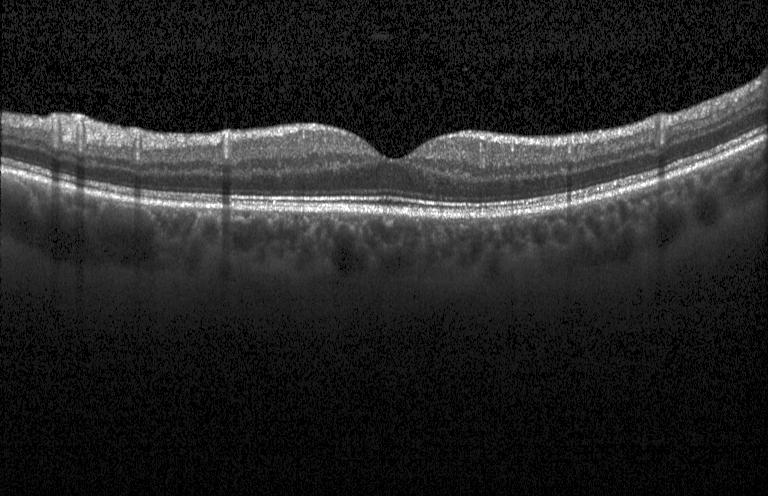

Retinal OCT cross-section showing no evidence of choroidal neovascularization, diabetic macular edema, or drusen.